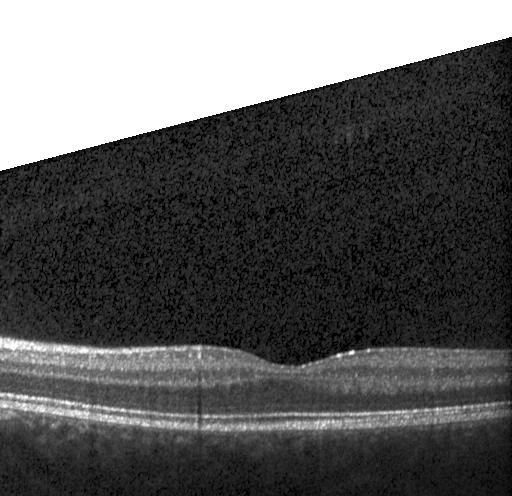 SD-OCT; OCT B-scan — Neither choroidal neovascularization, diabetic macular edema, nor drusen.